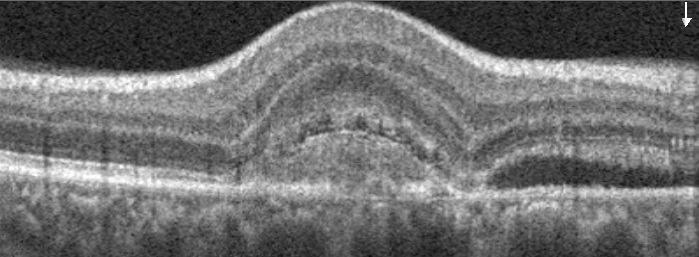
This B-scan demonstrates age-related macular degeneration (AMD).